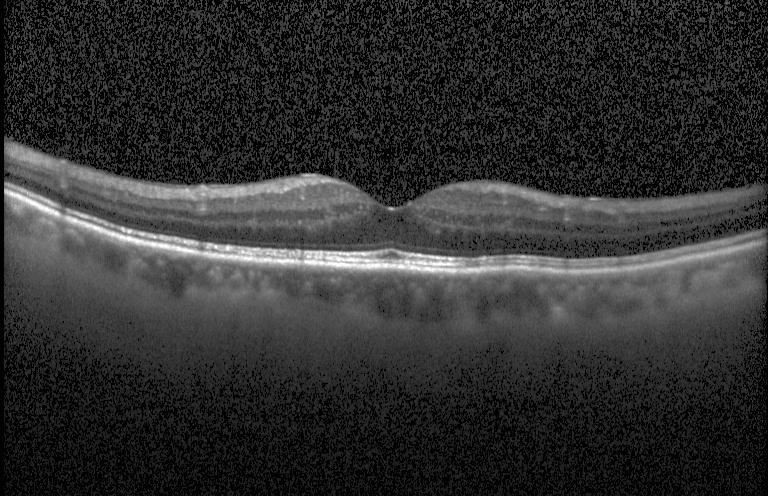
Retinal OCT B-scan. SD-OCT.
Impression: no choroidal neovascularization, no diabetic macular edema, and no drusen.